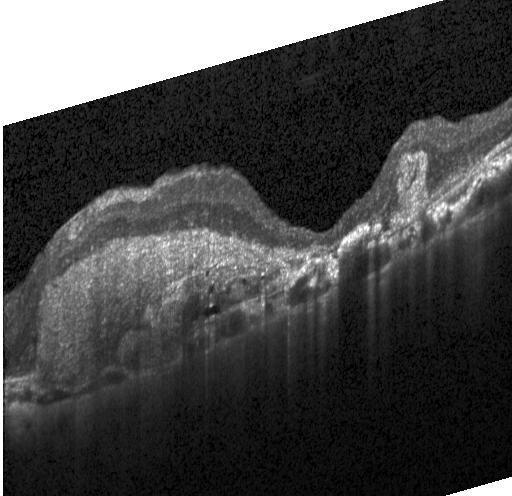

OCT B-scan
Dx: a choroidal neovascular membrane.